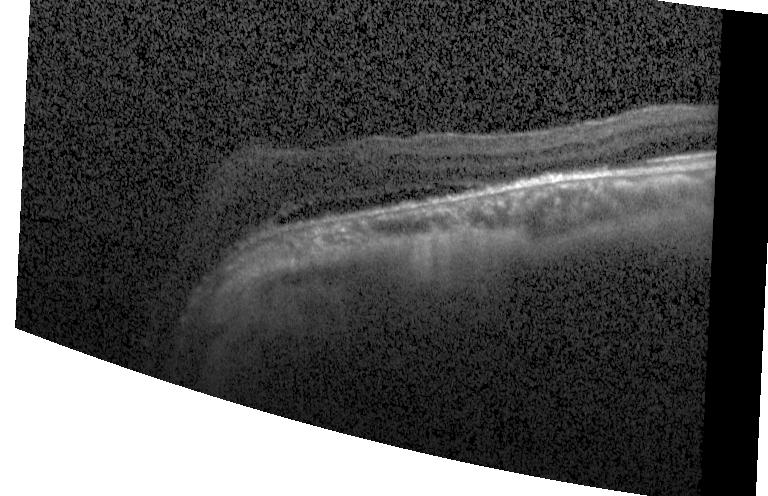

Spectral-domain OCT B-scan: choroidal neovascularization.